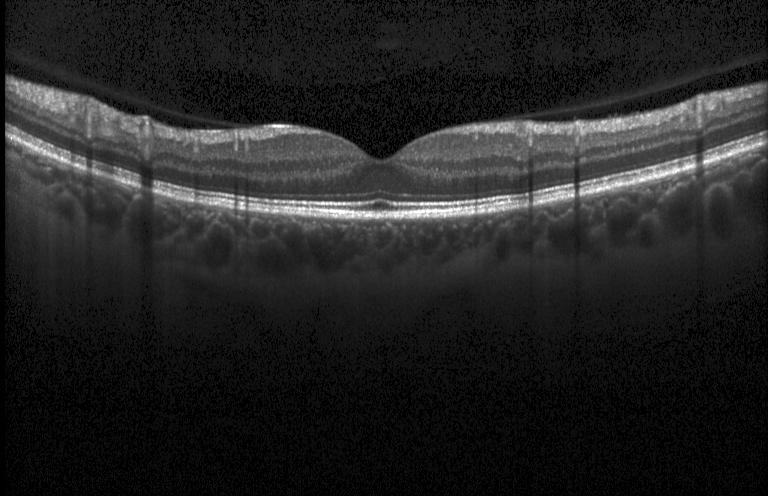
Horizontal scan through the fovea · OCT B-scan · SD-OCT.
Finding: no evidence of choroidal neovascularization, diabetic macular edema, or drusen.